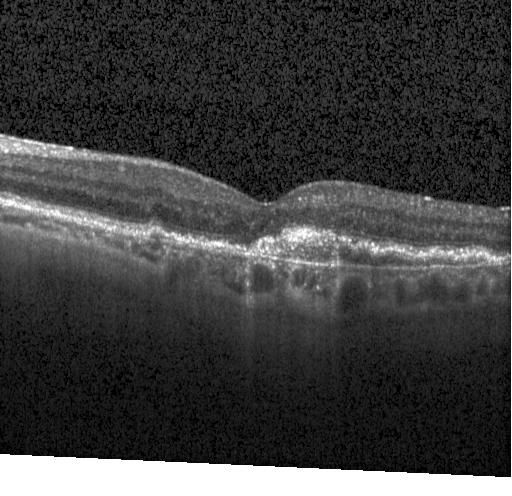

Retinal OCT cross-section — Impression: CNV.